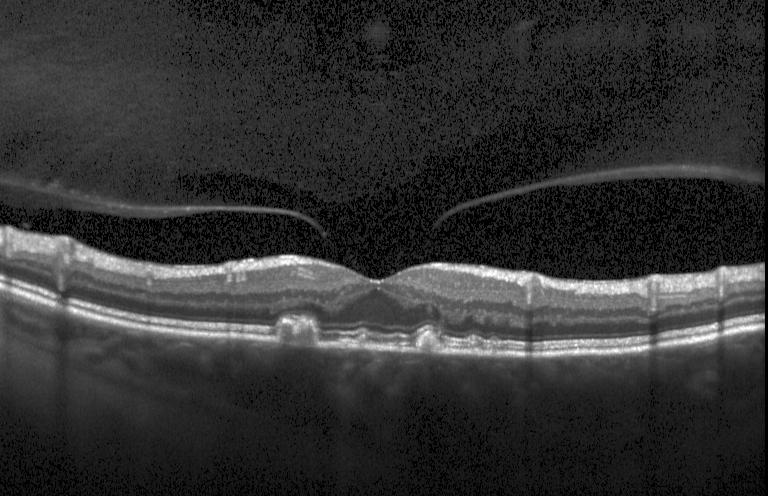

Horizontal scan through the fovea, Heidelberg Spectralis, OCT line scan, spectral-domain optical coherence tomography. This B-scan demonstrates multiple drusen.